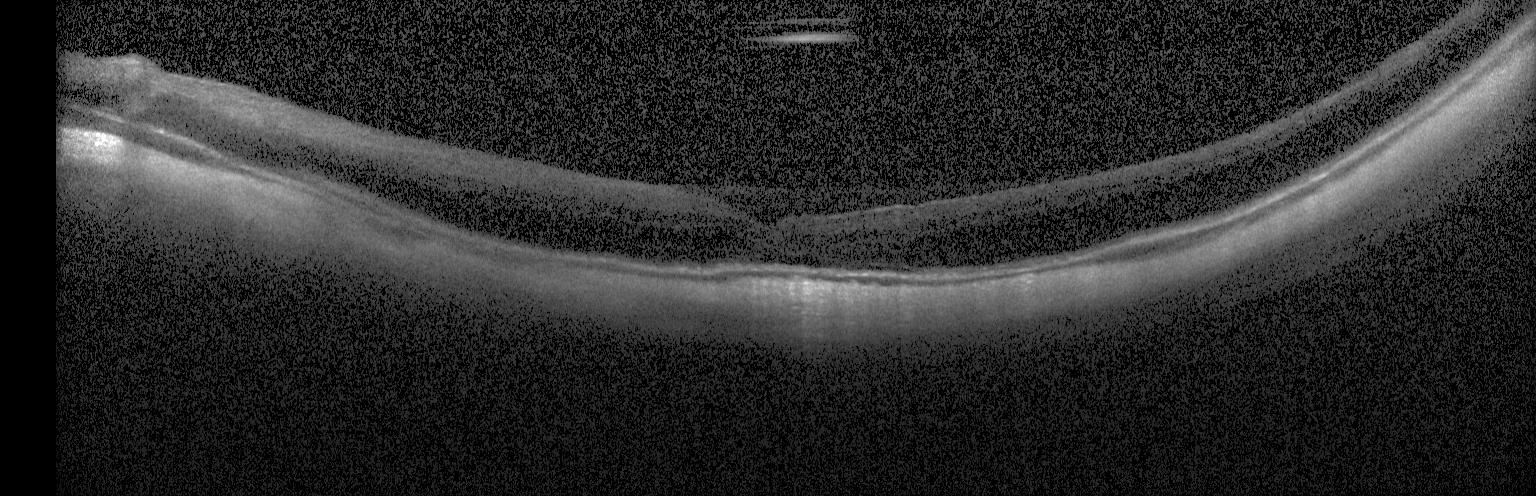 Macular scan; instrument: Heidelberg Spectralis; retinal OCT B-scan; spectral-domain OCT.
Diagnosis: diabetic macular edema (DME).